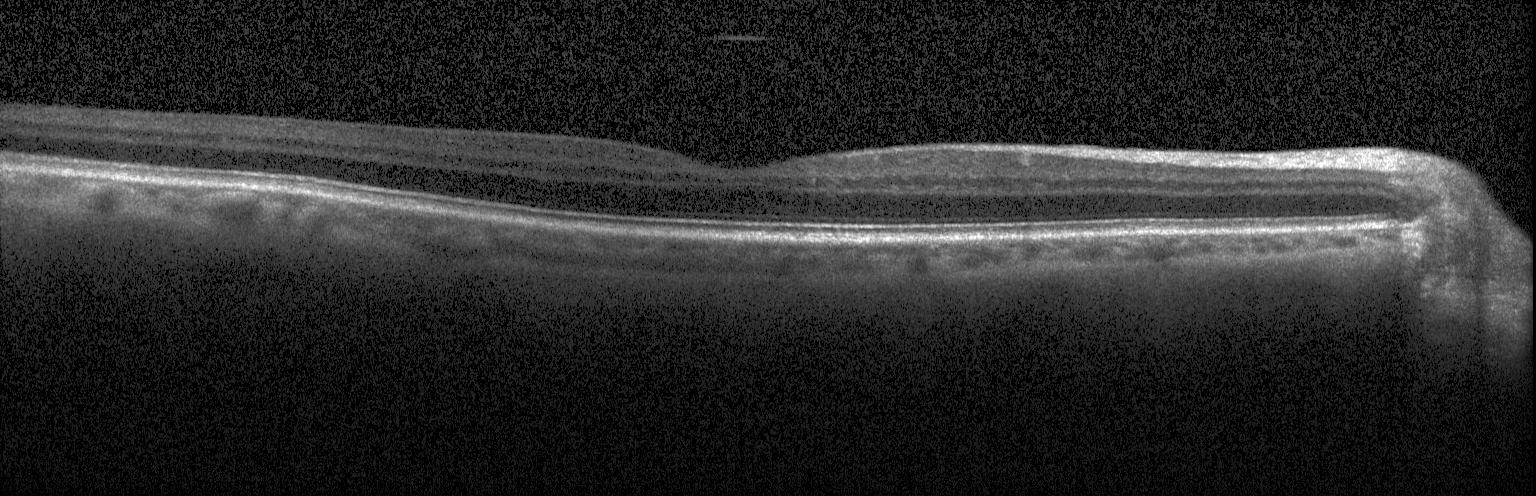 Impression: no CNV, DME, or drusen.